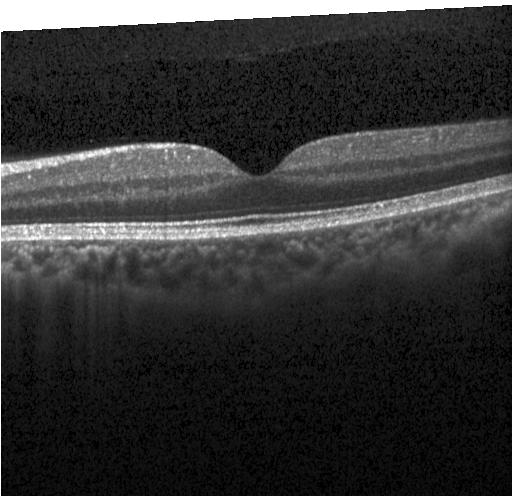 Instrument: Heidelberg Spectralis · spectral-domain OCT · retinal OCT cross-section
The scan shows no CNV, no DME, and no drusen.